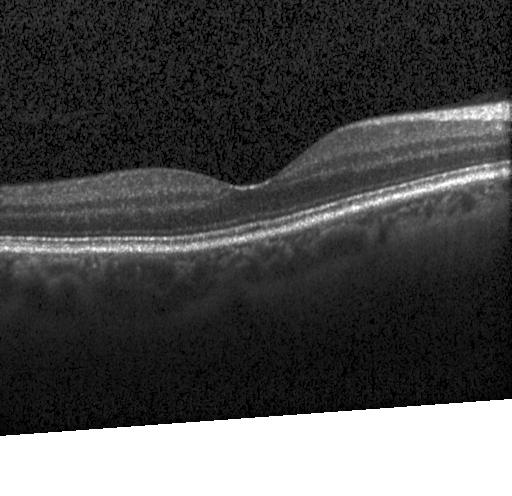

Acquired on a Heidelberg Spectralis. Optical coherence tomography scan — Assessment: no choroidal neovascularization, diabetic macular edema, or drusen.